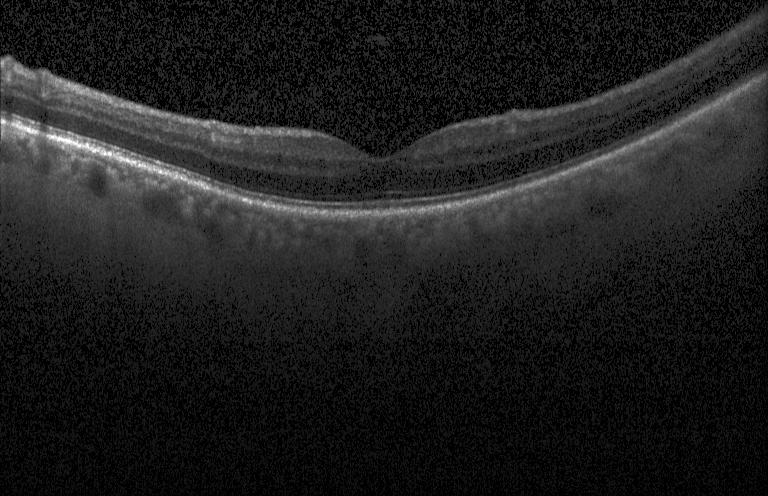 Instrument: Heidelberg Spectralis · centered on the fovea · OCT B-scan · SD-OCT
Assessment: no choroidal neovascularization, diabetic macular edema, or drusen.